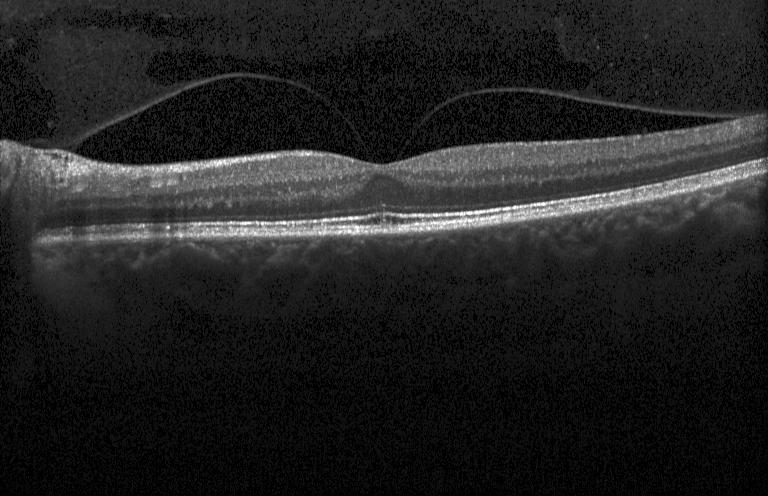 Heidelberg Spectralis, spectral-domain OCT, OCT B-scan — The scan shows no choroidal neovascularization, no diabetic macular edema, and no drusen.